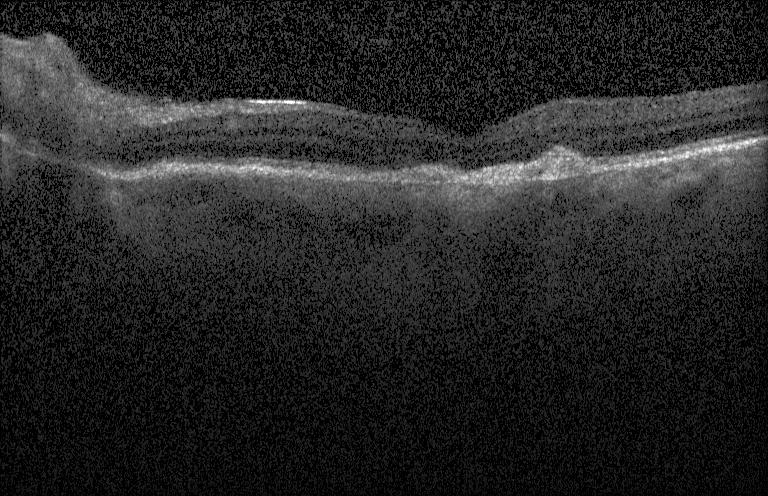 OCT finding: a choroidal neovascular membrane.